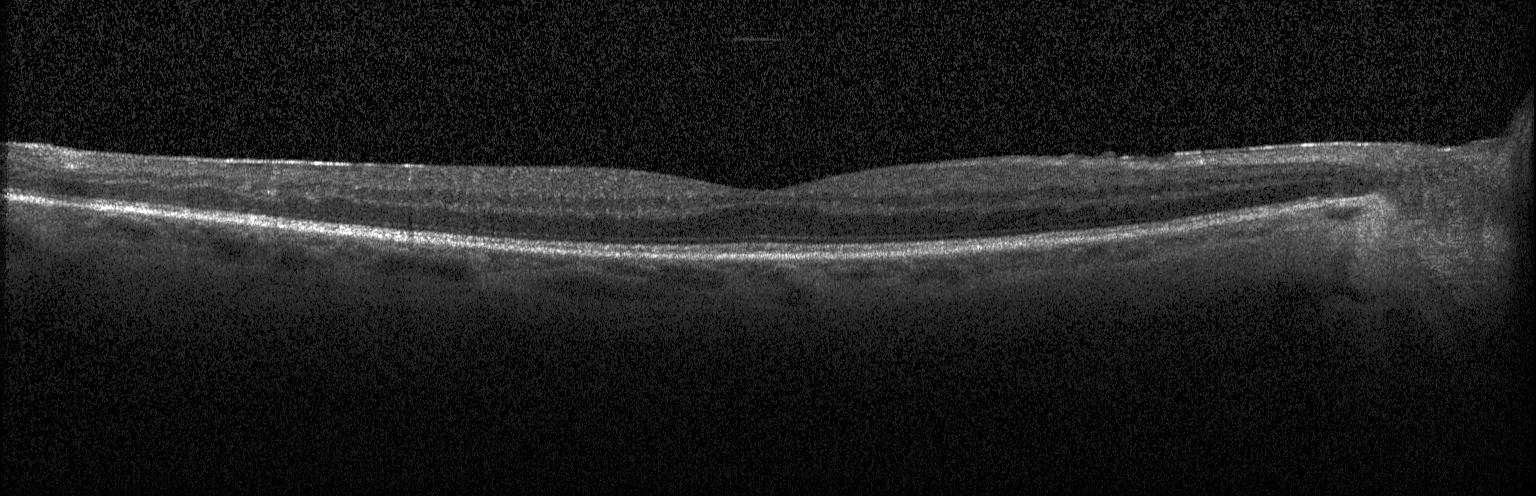

SD-OCT. Fovea-centered. Acquired on a Heidelberg Spectralis. OCT B-scan — Neither CNV, DME, nor drusen.